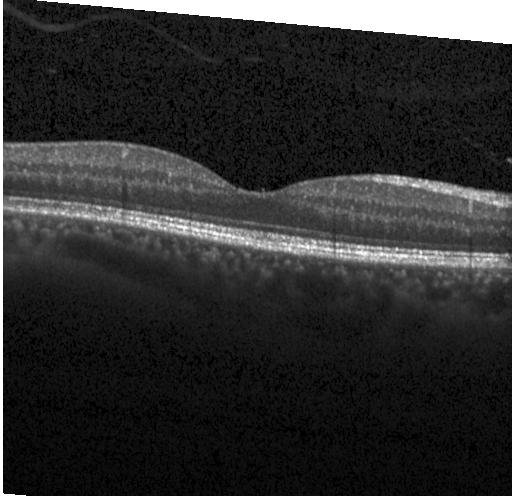
No evidence of choroidal neovascularization, diabetic macular edema, or drusen.